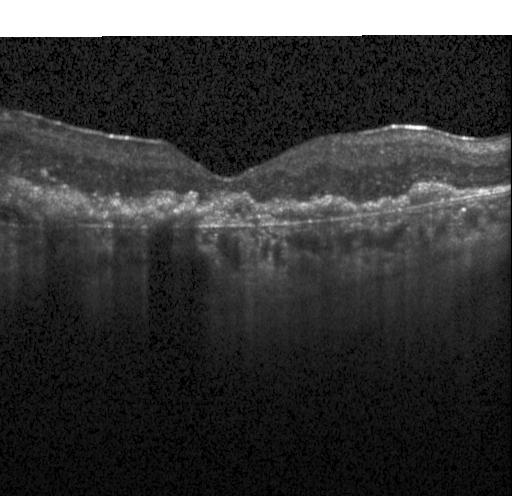 This B-scan demonstrates a choroidal neovascular membrane.